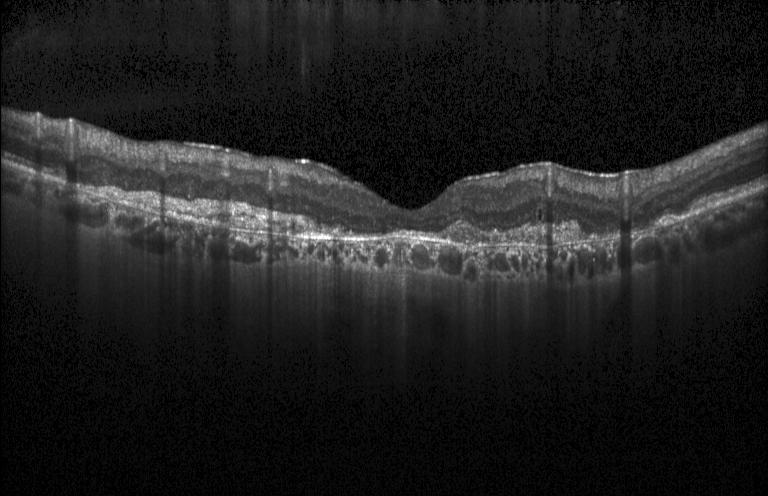 This B-scan demonstrates a choroidal neovascular membrane.